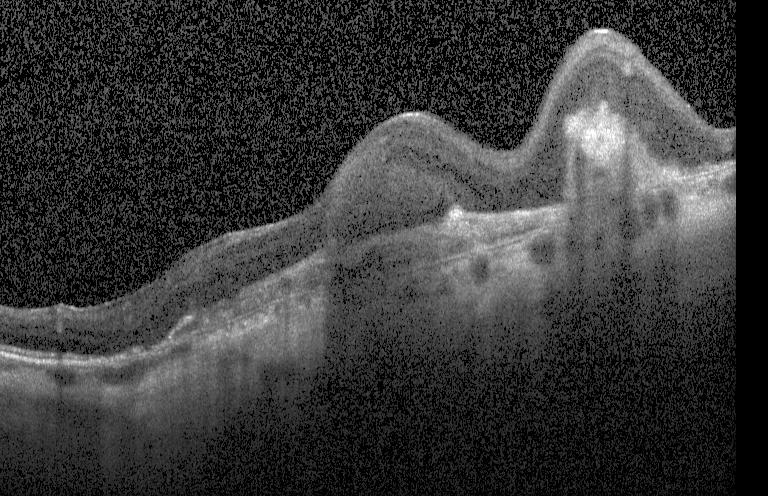
Optical coherence tomography B-scan — Diagnosis: a choroidal neovascular membrane.